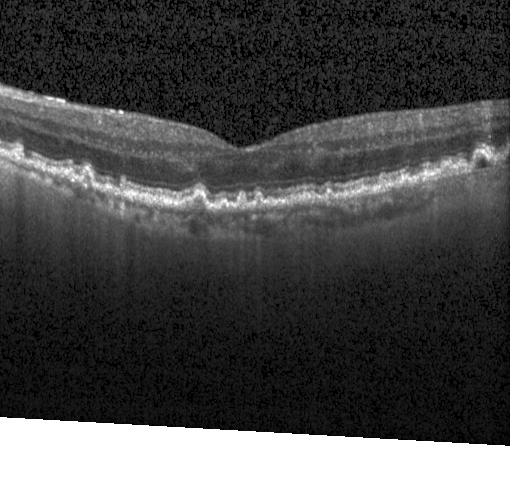

OCT B-scan; instrument: Heidelberg Spectralis — Dx: multiple drusen.